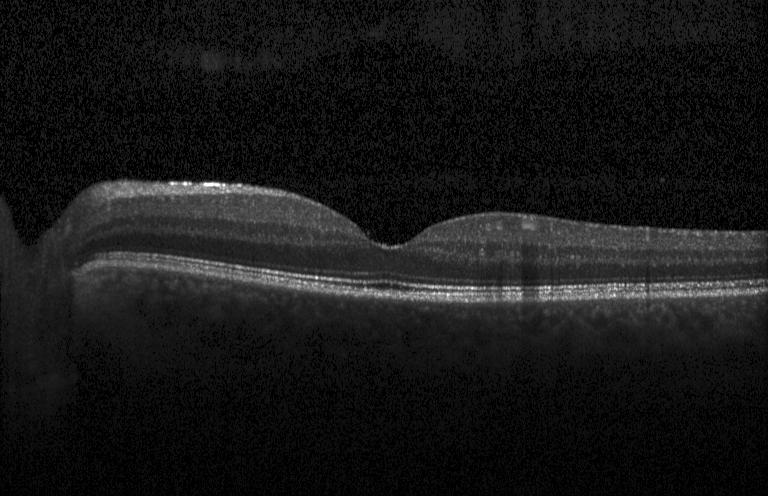
Heidelberg Spectralis OCT system; retinal OCT cross-section; spectral-domain optical coherence tomography; macular scan. The scan shows no CNV, no DME, and no drusen.